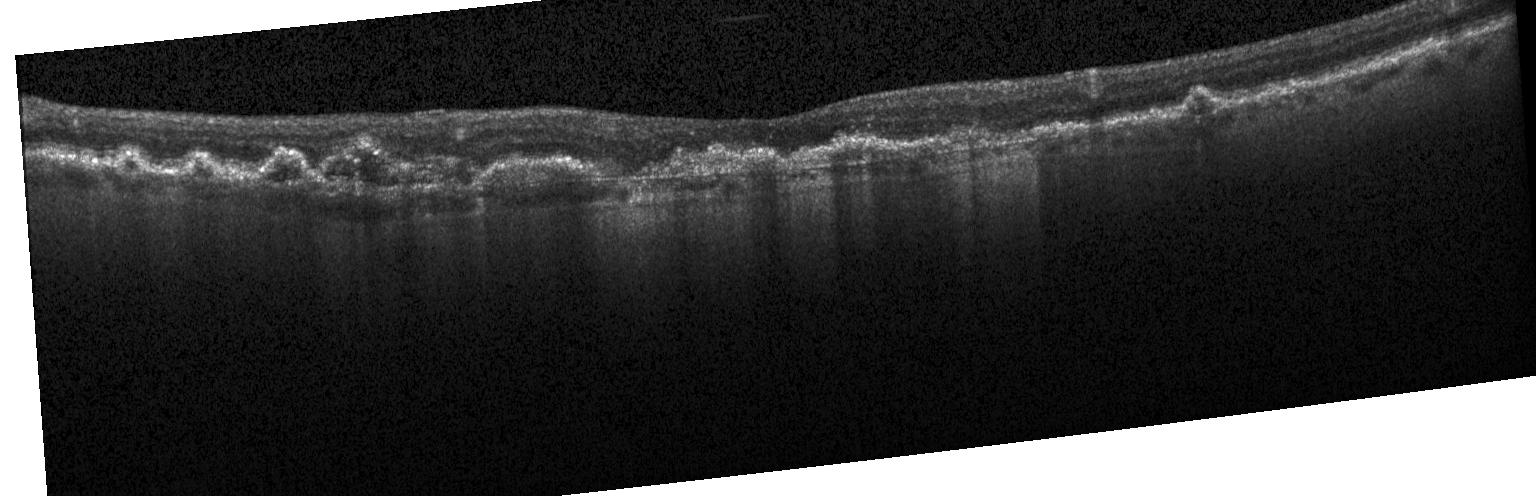 Retinal OCT B-scan.
Finding: a choroidal neovascular membrane.